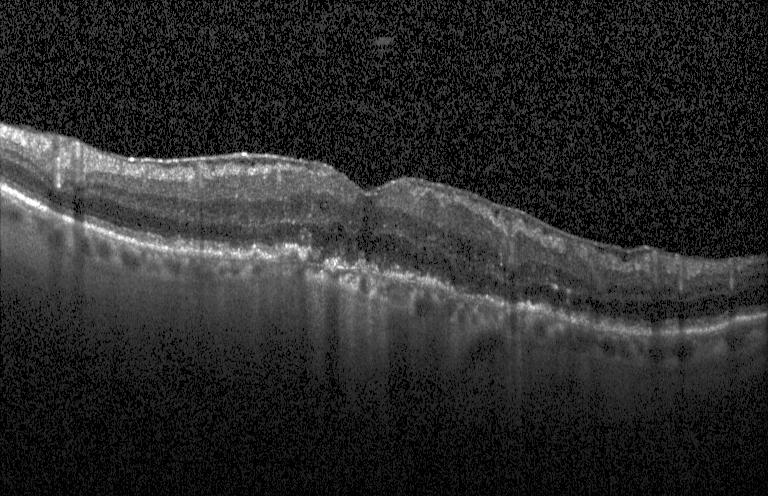

Optical coherence tomography scan. Macular scan — The scan shows CNV.